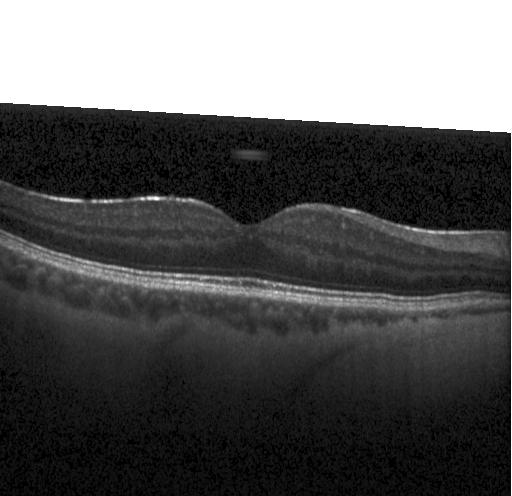
Impression: no choroidal neovascularization, no diabetic macular edema, and no drusen.